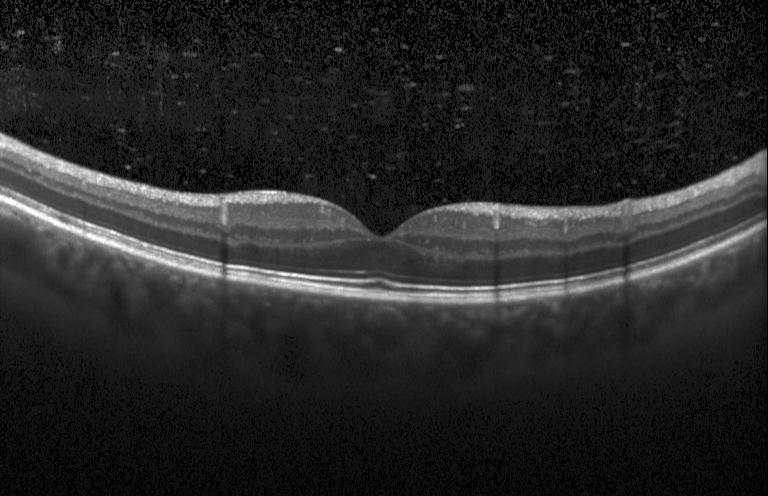 OCT scan showing no evidence of choroidal neovascularization, diabetic macular edema, or drusen.